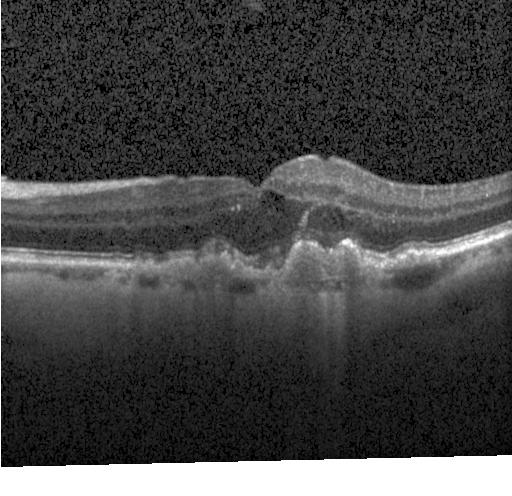
OCT line scan. Spectral-domain OCT.
The scan shows choroidal neovascularization.